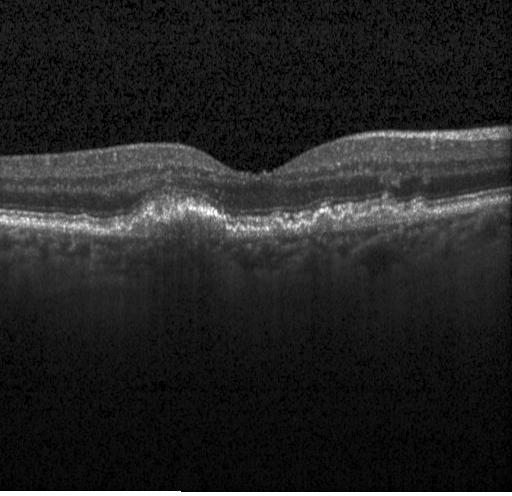

Retinal OCT B-scan
Assessment: sub-RPE drusenoid deposits.